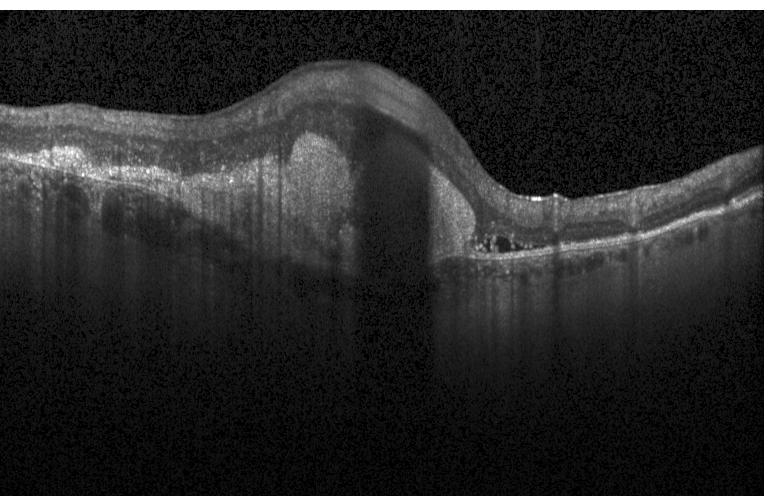
SD-OCT; Heidelberg Spectralis OCT system; OCT B-scan — Impression: a choroidal neovascular membrane.